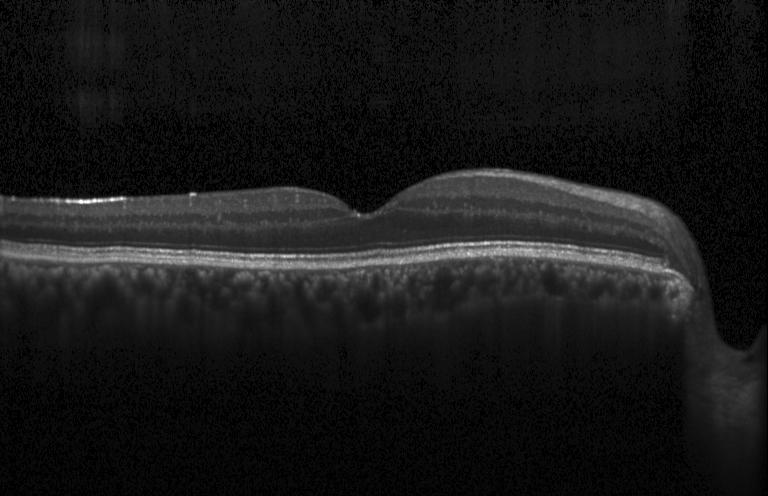
Centered on the fovea · optical coherence tomography B-scan · Heidelberg Spectralis OCT system · spectral-domain OCT. Finding: no CNV, no DME, and no drusen.